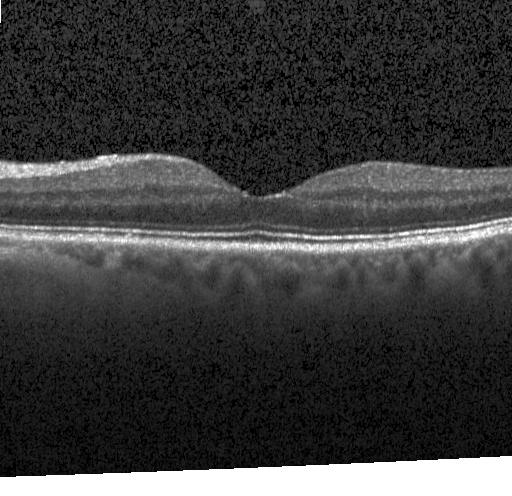

Heidelberg Spectralis OCT system; OCT line scan; spectral-domain optical coherence tomography
Finding: neither choroidal neovascularization, diabetic macular edema, nor drusen.